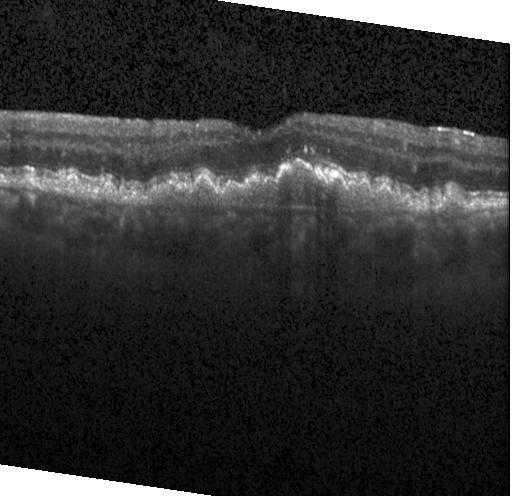
OCT B-scan, spectral-domain optical coherence tomography, centered on the fovea. Finding: a choroidal neovascular membrane.